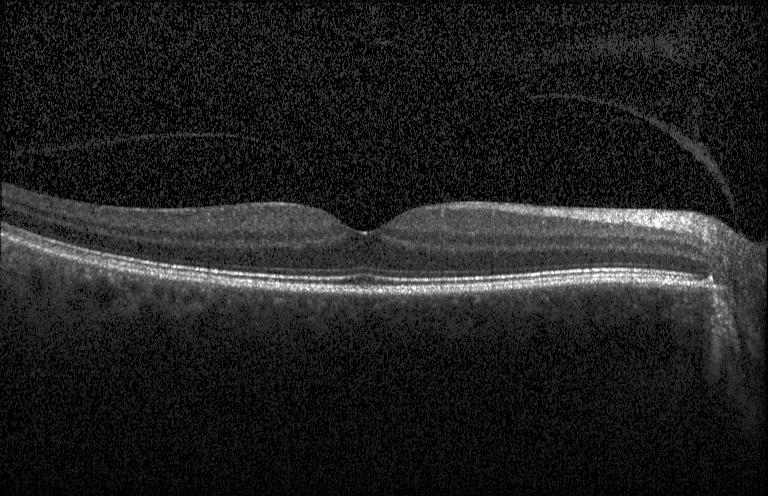 OCT B-scan · SD-OCT
Diagnosis: no choroidal neovascularization, diabetic macular edema, or drusen.